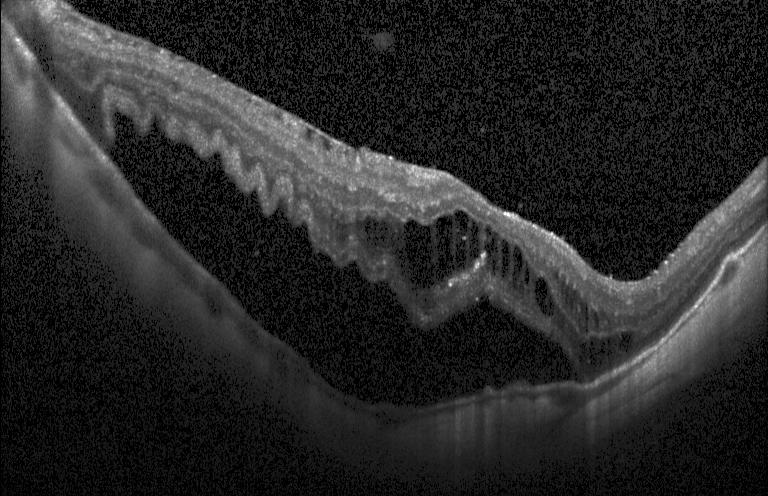 Spectral-domain OCT B-scan: CNV.